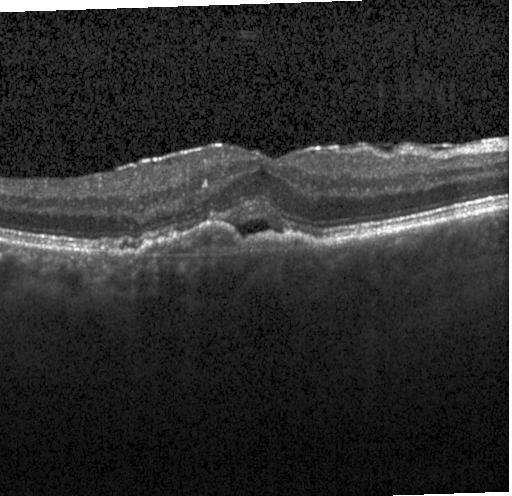
OCT finding: a choroidal neovascular membrane.